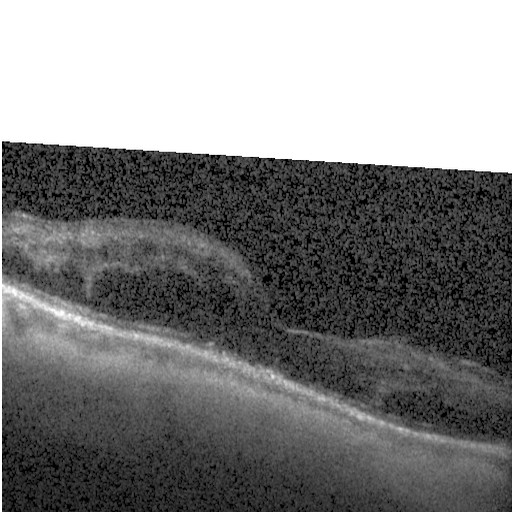
Retinal OCT cross-section
Diagnosis: diabetic macular edema.